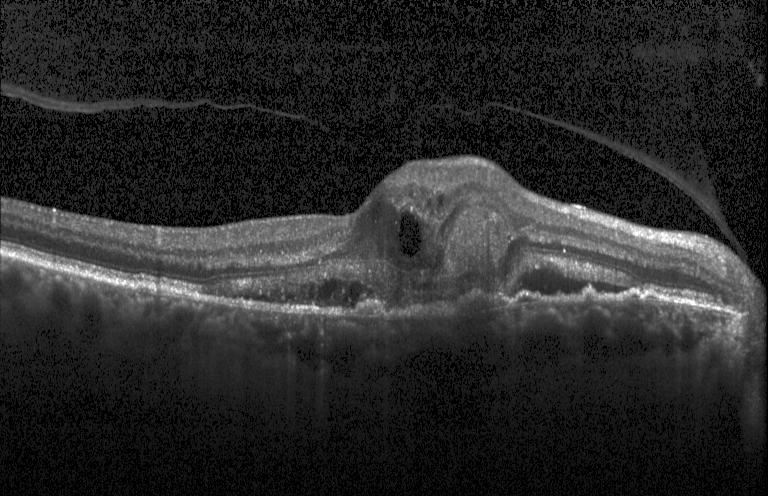

Retinal OCT B-scan — CNV.